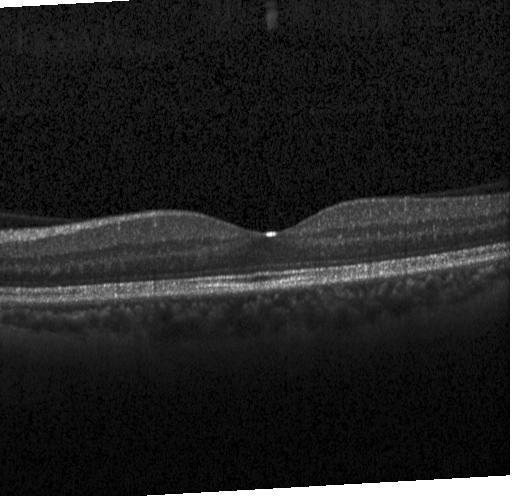 Impression: no choroidal neovascularization, diabetic macular edema, or drusen.